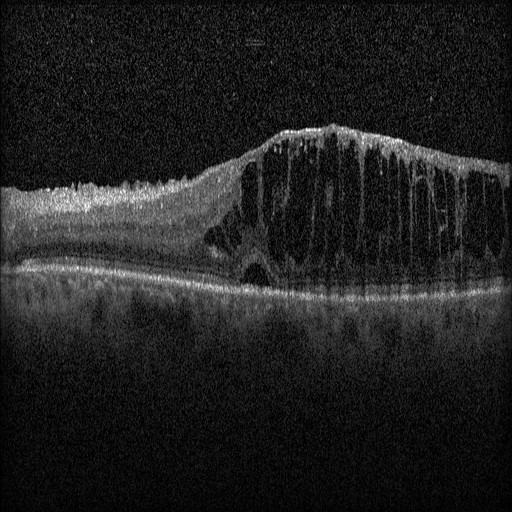 OCT finding: diabetic macular edema (DME).